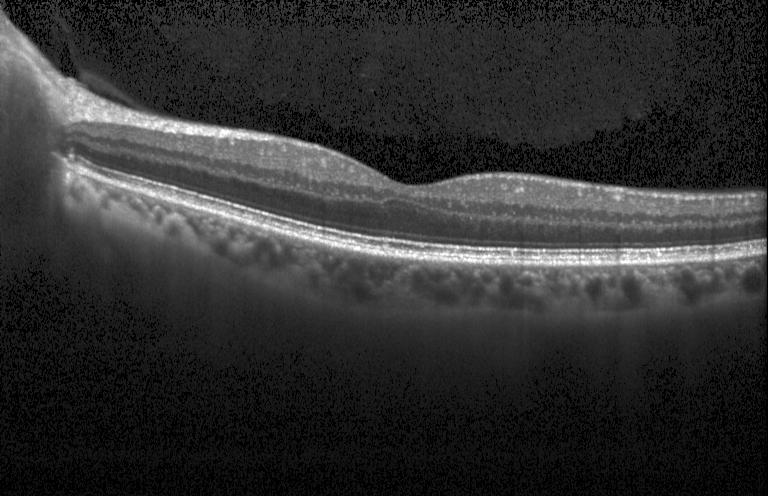
Impression: neither choroidal neovascularization, diabetic macular edema, nor drusen.